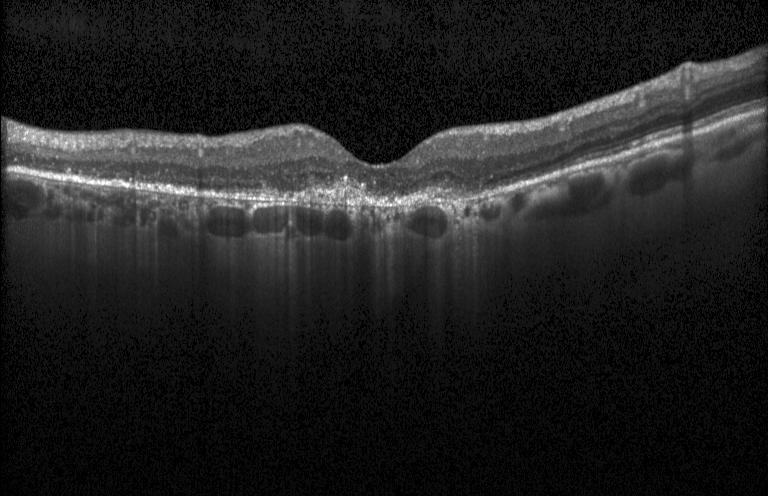

Spectral-domain optical coherence tomography; optical coherence tomography B-scan. This B-scan demonstrates choroidal neovascularization (CNV).